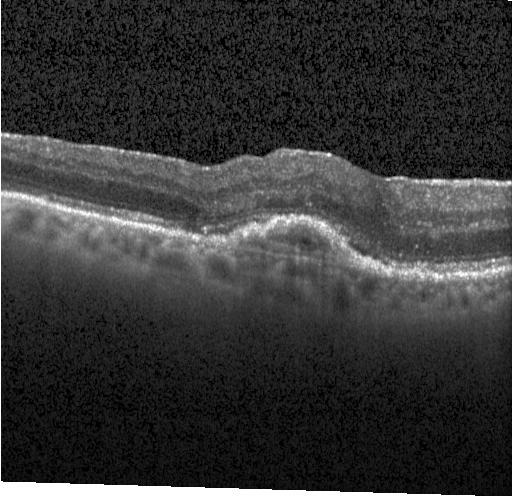 Optical coherence tomography B-scan · fovea-centered · instrument: Heidelberg Spectralis · SD-OCT. Finding: choroidal neovascularization.